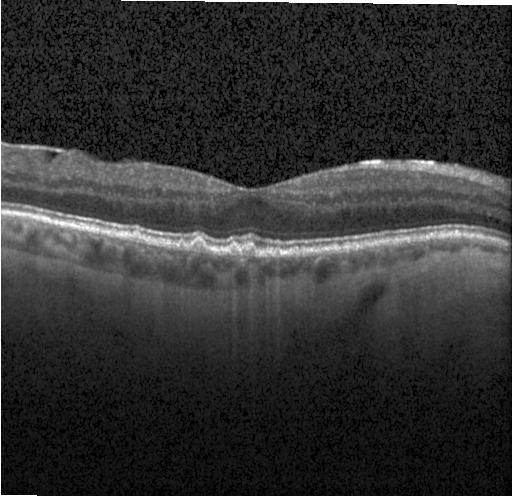 OCT finding: drusen.